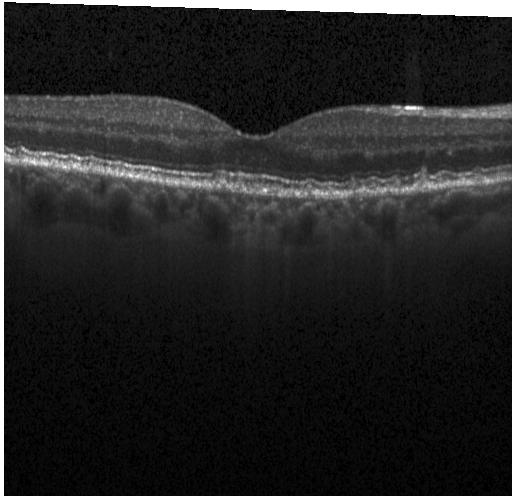
Drusen.